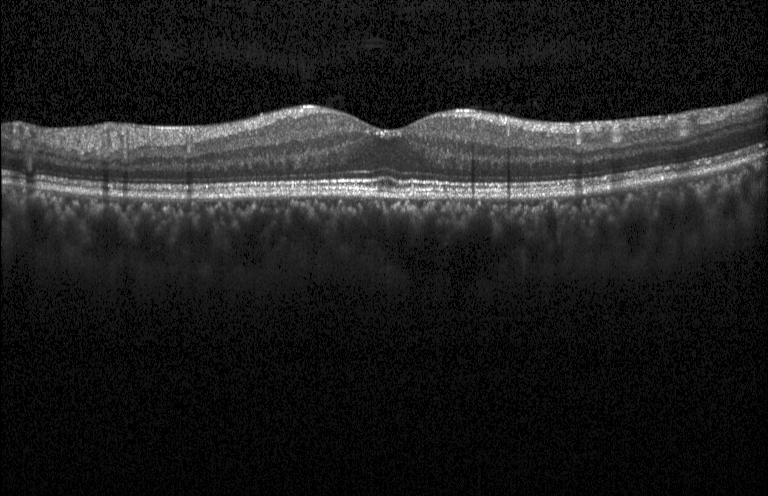

Heidelberg Spectralis OCT system. Optical coherence tomography scan. SD-OCT. Centered on the fovea
This B-scan demonstrates no evidence of CNV, DME, or drusen.